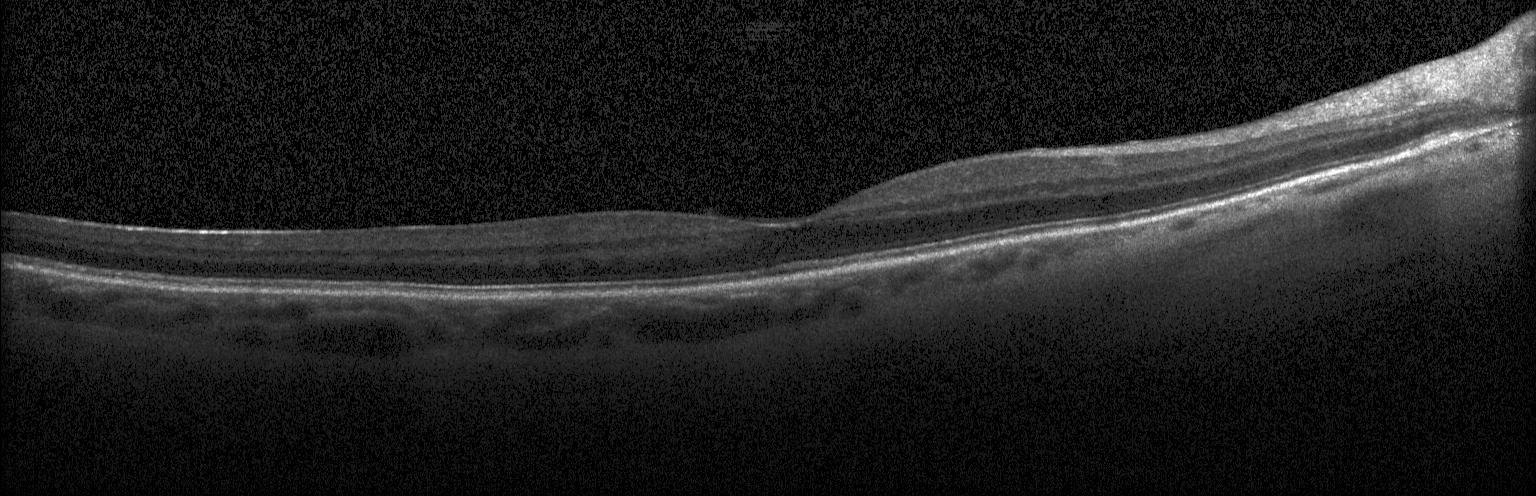

Heidelberg Spectralis OCT system, spectral-domain OCT, macular scan, retinal OCT B-scan
Finding: no evidence of choroidal neovascularization, diabetic macular edema, or drusen.